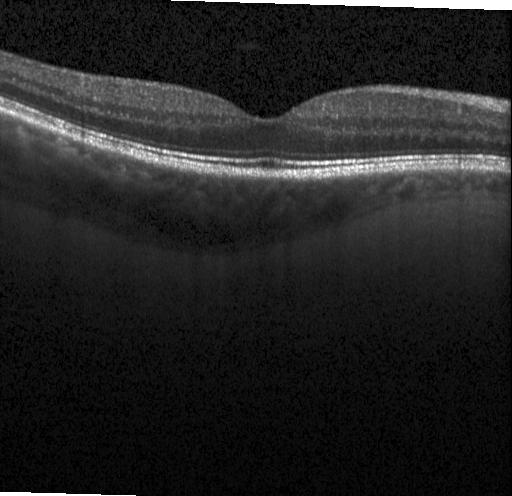
Through the macula; optical coherence tomography scan; acquired on a Heidelberg Spectralis; spectral-domain OCT
Diagnosis: no CNV, DME, or drusen.